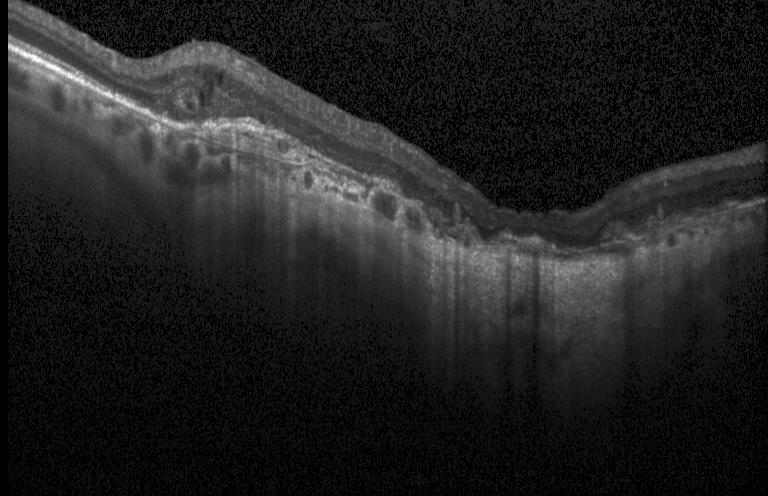
Spectral-domain OCT B-scan: CNV.